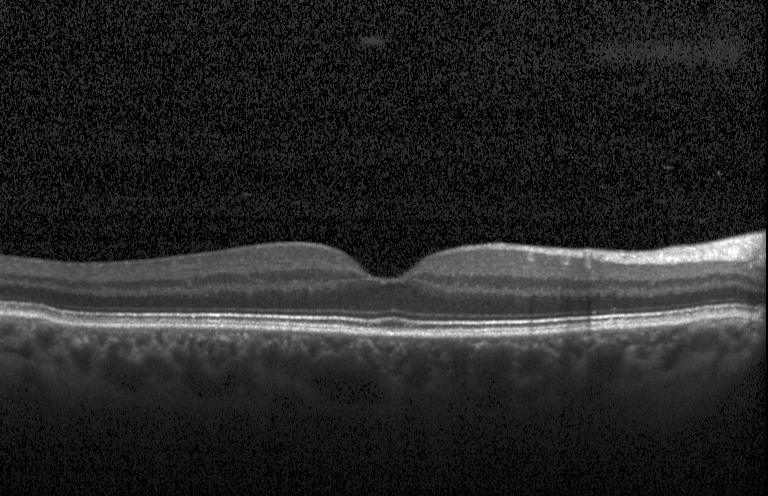 SD-OCT · OCT line scan
Impression: neither choroidal neovascularization, diabetic macular edema, nor drusen.